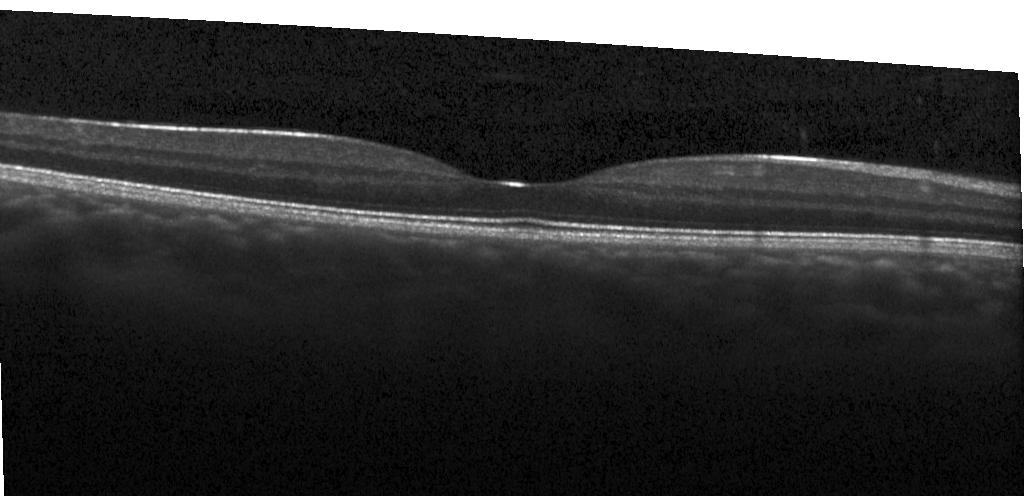 Diagnosis: no choroidal neovascularization, diabetic macular edema, or drusen.